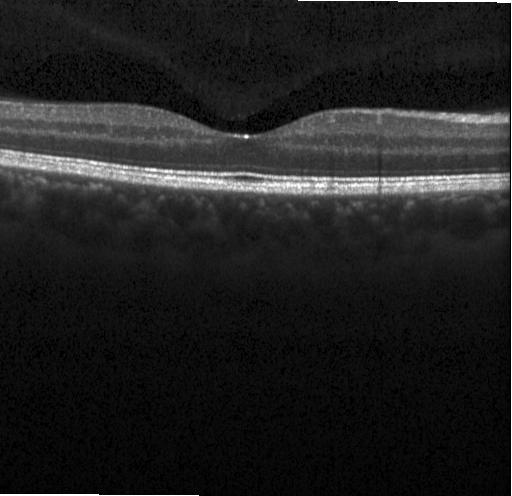

Macular OCT: no evidence of choroidal neovascularization, diabetic macular edema, or drusen.